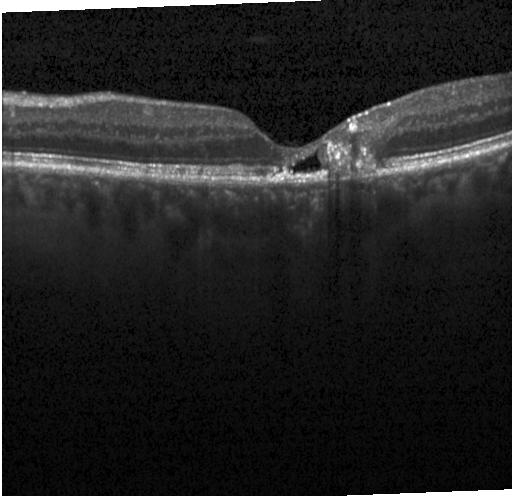

Spectral-domain OCT, OCT B-scan
Macular OCT: a choroidal neovascular membrane.